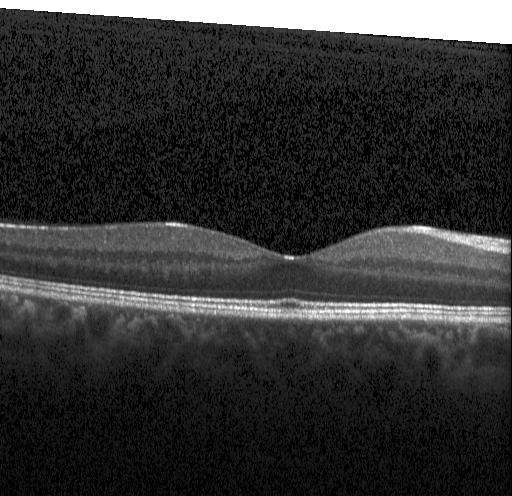 Finding: no choroidal neovascularization, diabetic macular edema, or drusen.